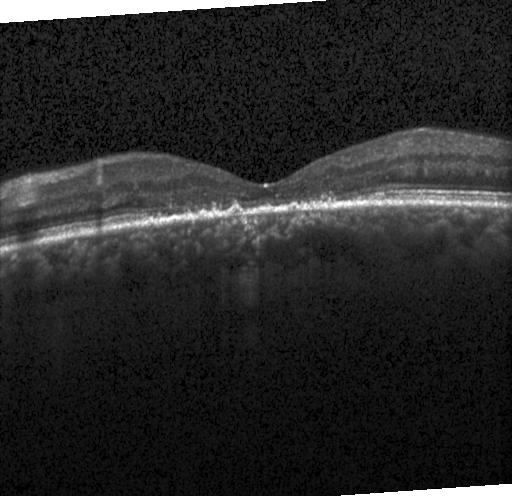 Finding: multiple drusen.